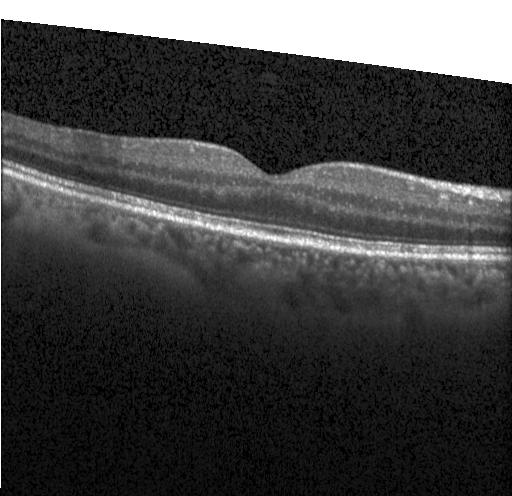

Macular scan; optical coherence tomography B-scan — Macular OCT: neither choroidal neovascularization, diabetic macular edema, nor drusen.